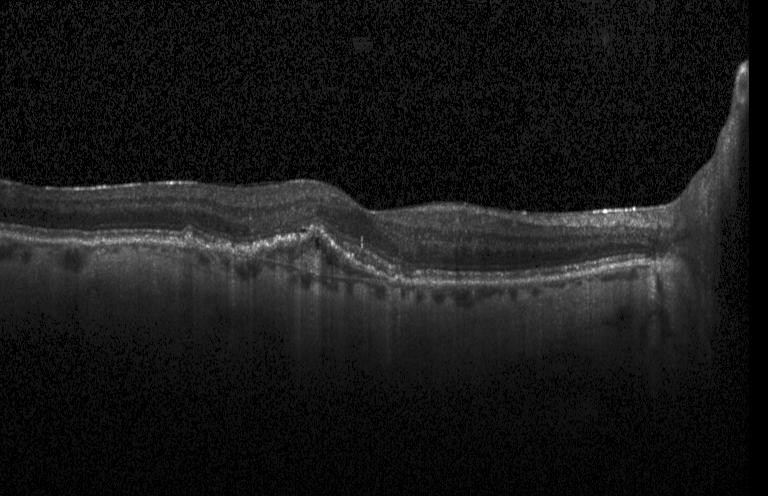

Optical coherence tomography B-scan — Finding: a choroidal neovascular membrane.